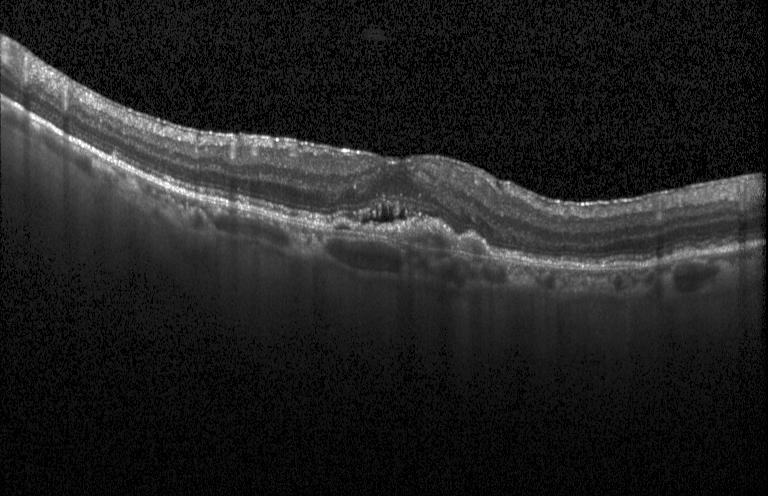

OCT B-scan. Through the macula.
Finding: CNV.